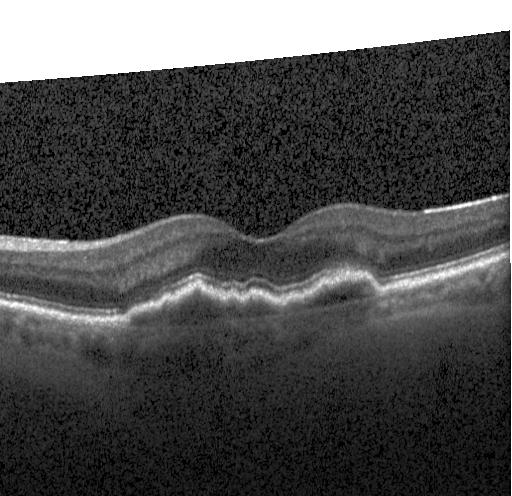

Retinal OCT cross-section · Heidelberg Spectralis OCT system
Finding: a choroidal neovascular membrane.